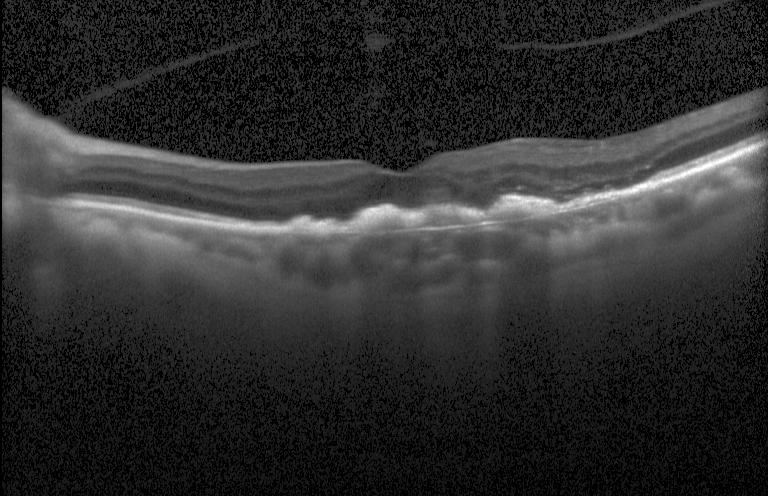 Horizontal scan through the fovea · acquired on a Heidelberg Spectralis · optical coherence tomography scan. Diagnosis: choroidal neovascularization (CNV).